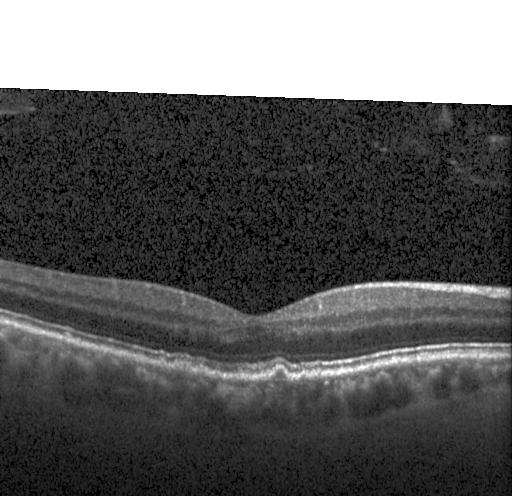
This B-scan demonstrates drusen.